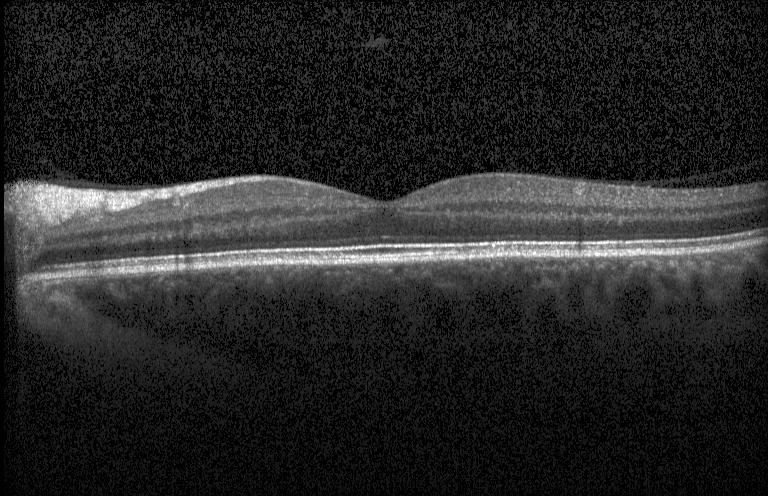

Spectral-domain OCT · retinal OCT B-scan — Finding: no CNV, no DME, and no drusen.